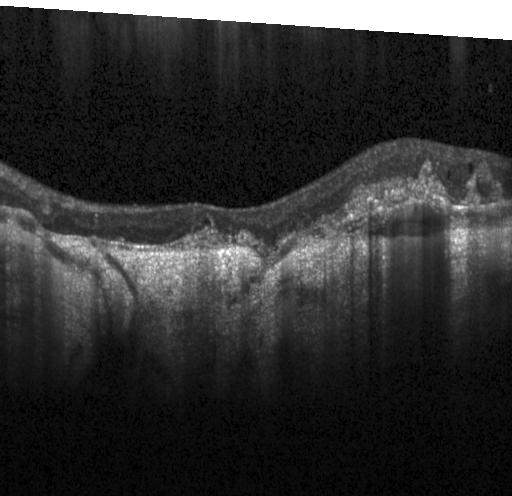

Diagnosis: CNV.